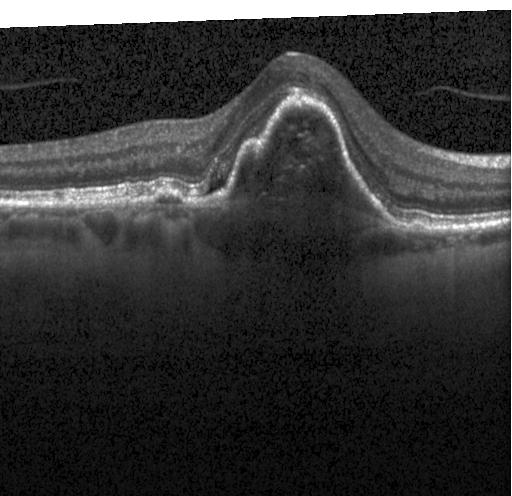 Spectral-domain optical coherence tomography · optical coherence tomography B-scan.
Dx: a choroidal neovascular membrane.